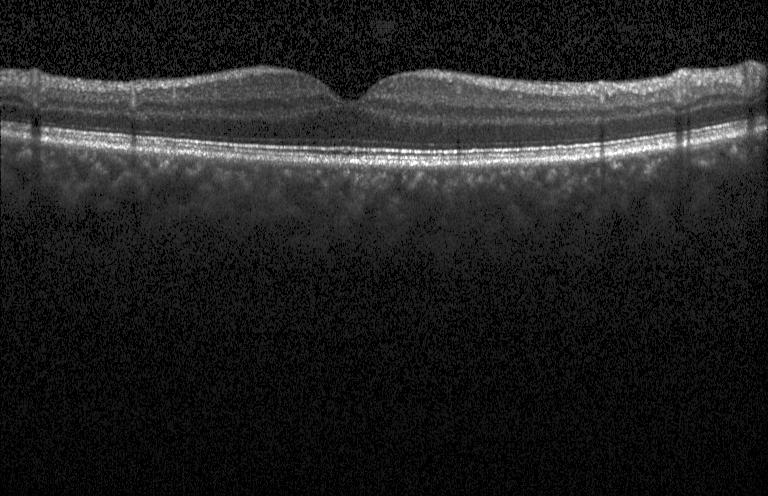 OCT B-scan. Centered on the fovea. Heidelberg Spectralis OCT system
The scan shows no choroidal neovascularization, diabetic macular edema, or drusen.